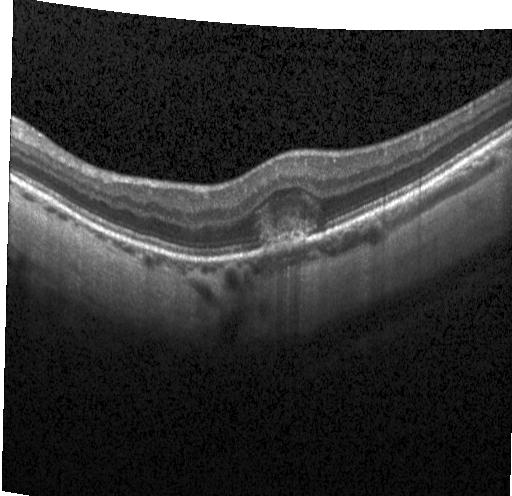

OCT B-scan, SD-OCT — This B-scan demonstrates choroidal neovascularization.